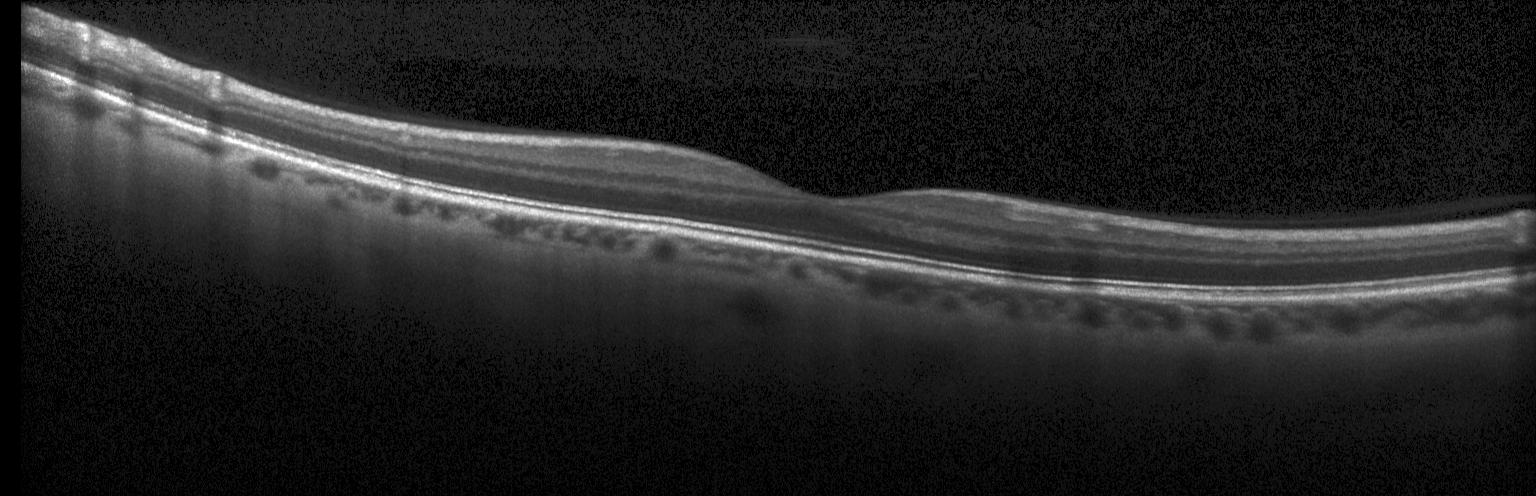
Retinal OCT B-scan — Diagnosis: no choroidal neovascularization, no diabetic macular edema, and no drusen.